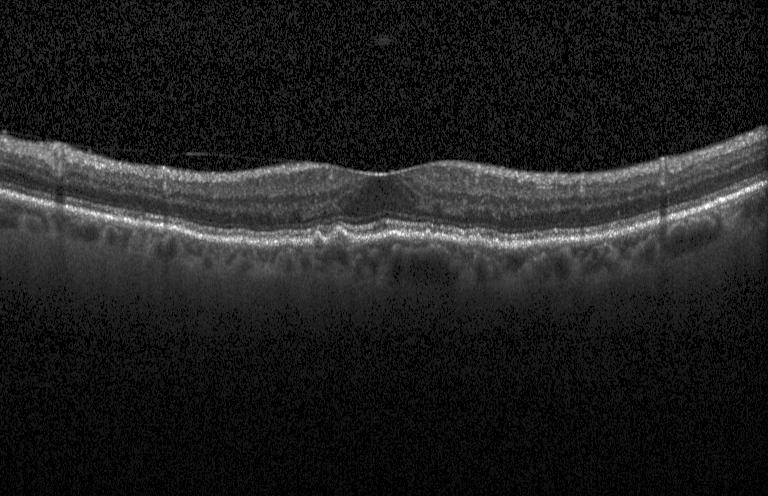 Macular scan; retinal OCT B-scan; Heidelberg Spectralis; spectral-domain OCT
Dx: sub-RPE drusenoid deposits.